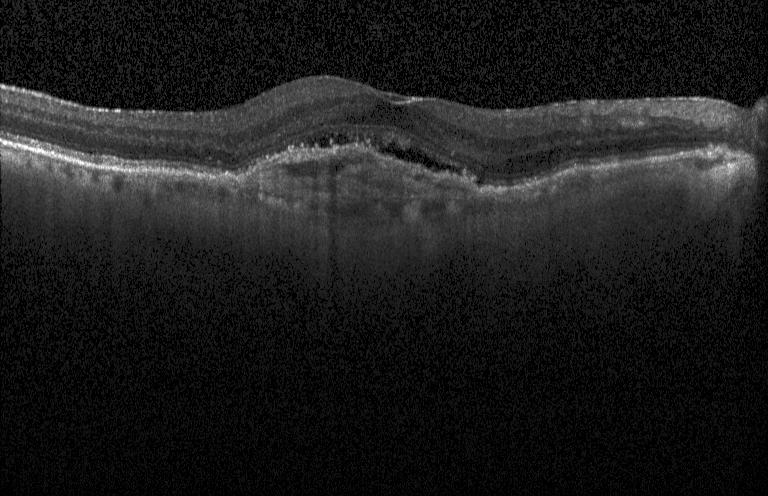 Heidelberg Spectralis · centered on the fovea · retinal OCT cross-section · SD-OCT
The scan shows a choroidal neovascular membrane.